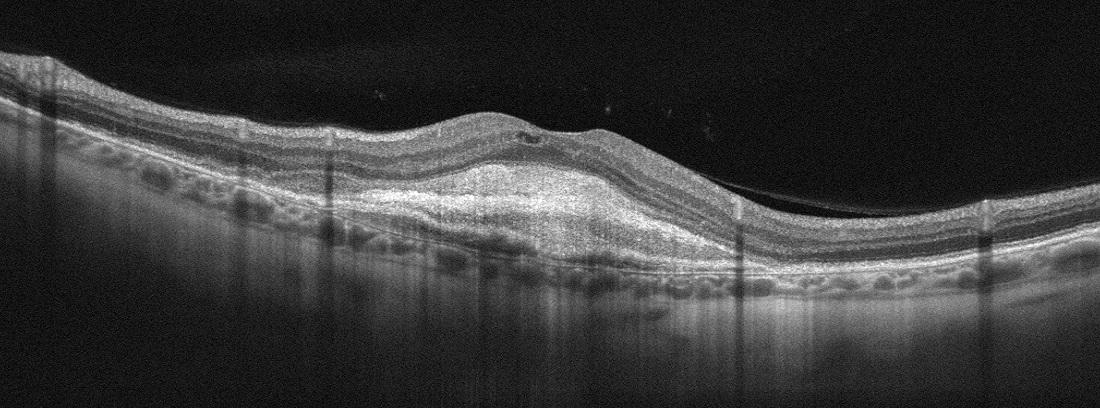

Impression: age-related macular degeneration (AMD).